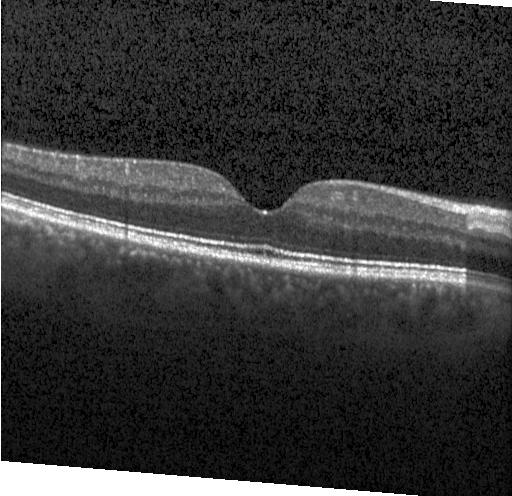

OCT B-scan · SD-OCT · Heidelberg Spectralis — This B-scan demonstrates no choroidal neovascularization, diabetic macular edema, or drusen.